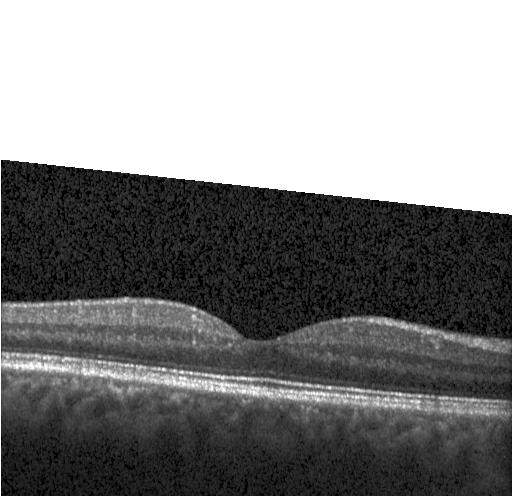
OCT B-scan
Diagnosis: no evidence of choroidal neovascularization, diabetic macular edema, or drusen.